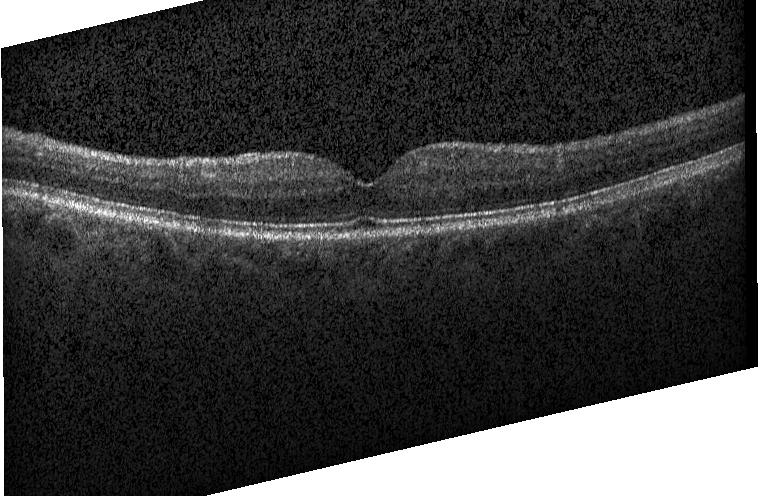 SD-OCT, optical coherence tomography scan — Impression: neither choroidal neovascularization, diabetic macular edema, nor drusen.